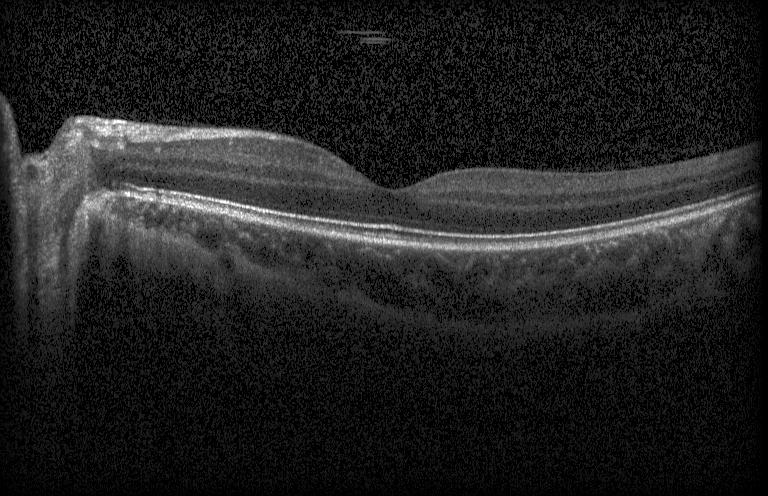

Horizontal scan through the fovea · spectral-domain OCT · optical coherence tomography scan — Impression: no evidence of choroidal neovascularization, diabetic macular edema, or drusen.